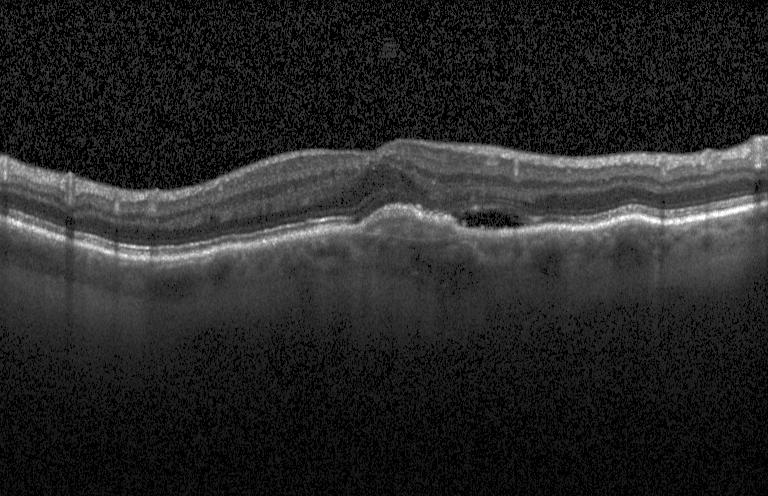
Instrument: Heidelberg Spectralis. SD-OCT. Centered on the fovea. OCT B-scan.
The scan shows a choroidal neovascular membrane.